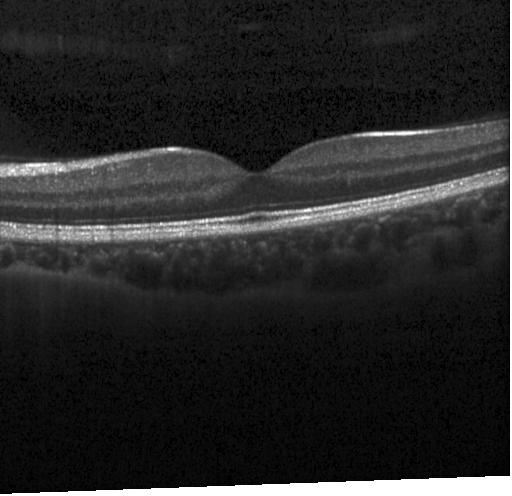 SD-OCT; macular scan; retinal OCT cross-section. Diagnosis: no CNV, no DME, and no drusen.